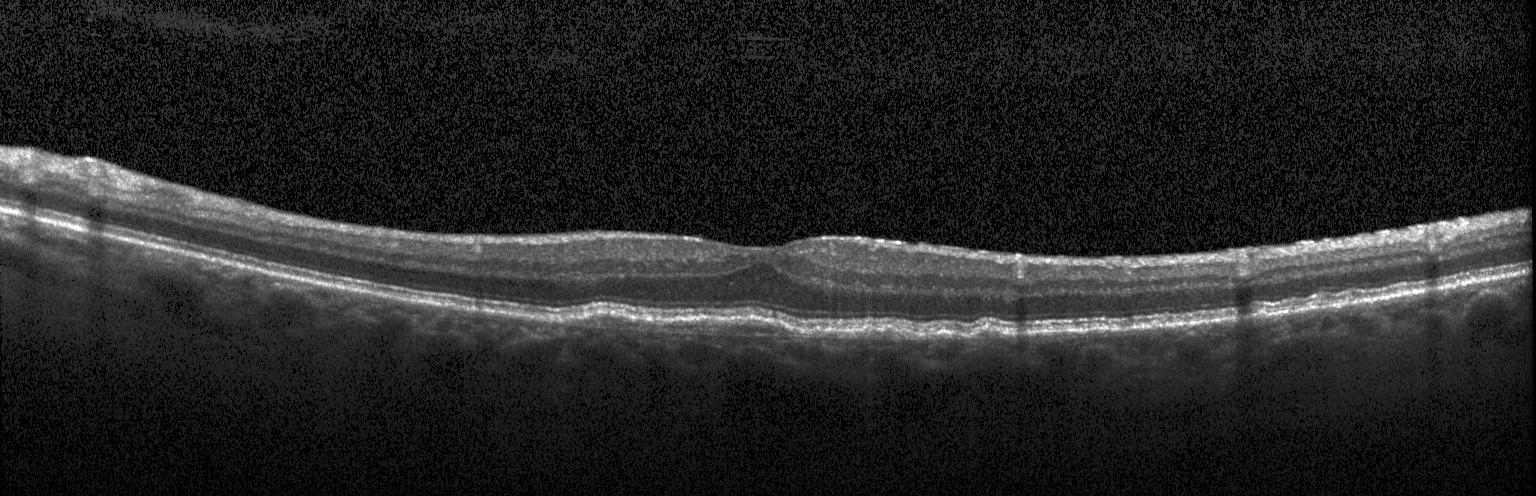 Dx: choroidal neovascularization.